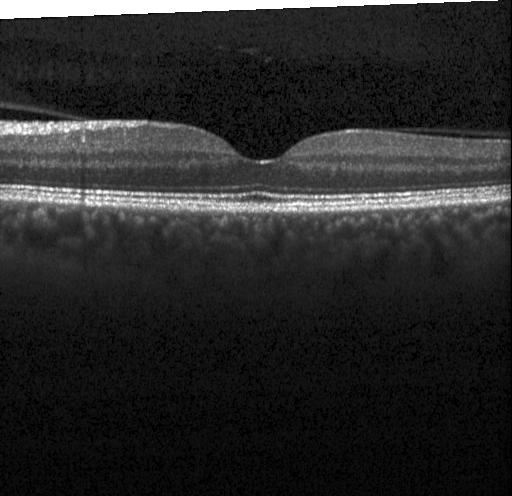
OCT line scan · spectral-domain optical coherence tomography · Heidelberg Spectralis · centered on the fovea. Impression: no evidence of choroidal neovascularization, diabetic macular edema, or drusen.